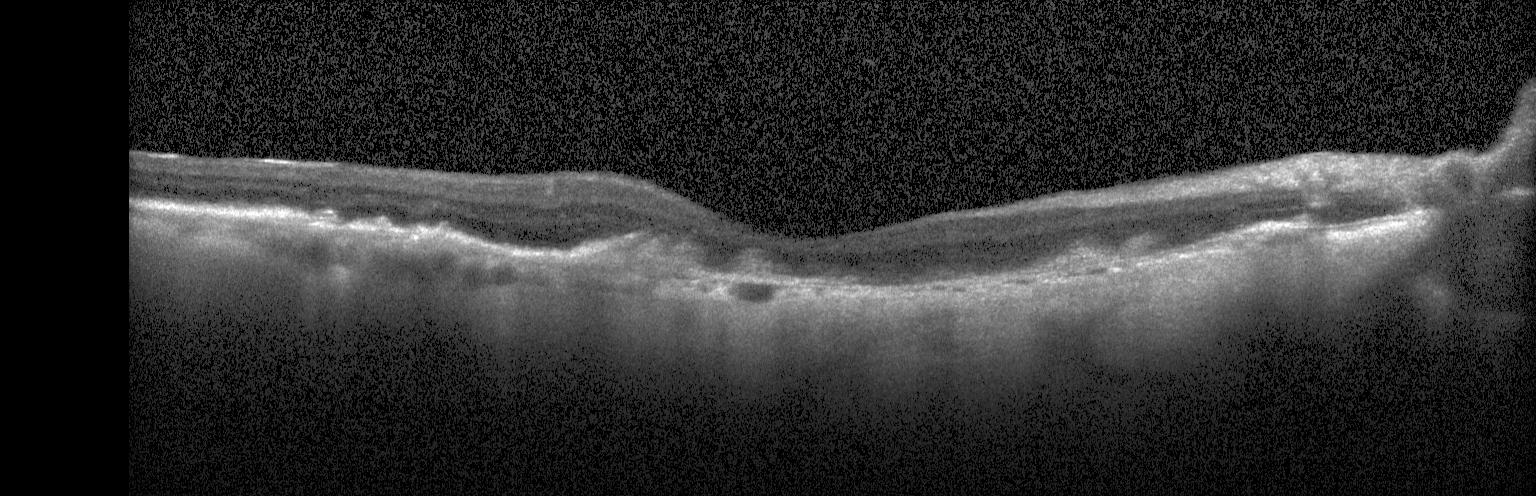

Retinal OCT B-scan. Through the macula
This B-scan demonstrates choroidal neovascularization (CNV).